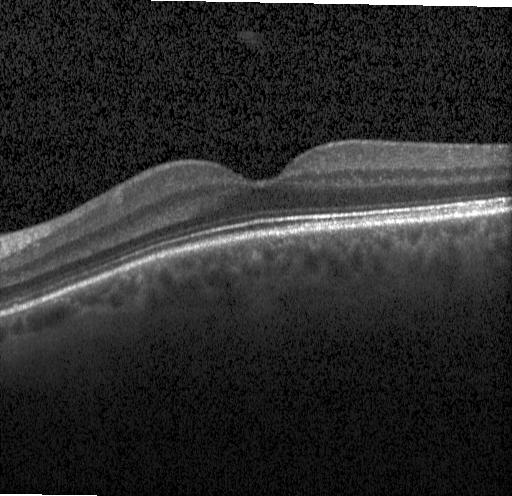

Macular OCT: no choroidal neovascularization, no diabetic macular edema, and no drusen.